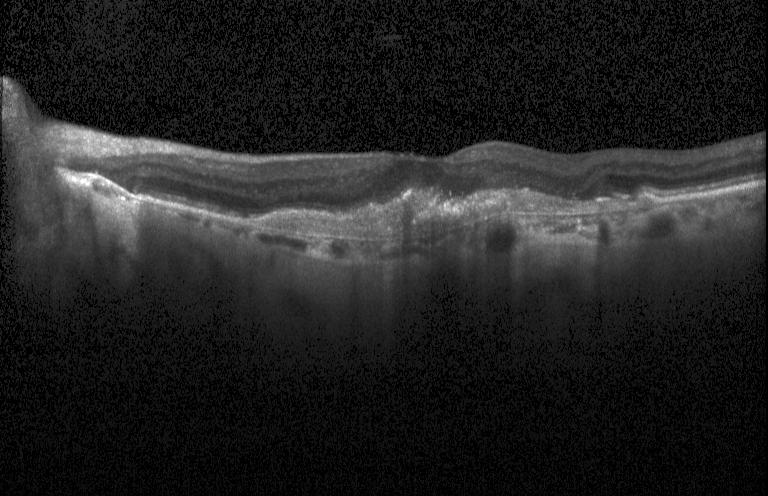
Retinal OCT B-scan — OCT finding: a choroidal neovascular membrane.